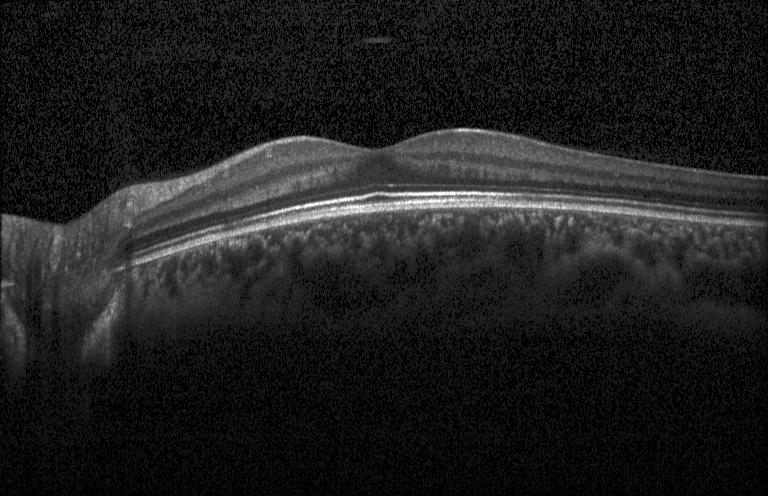

Heidelberg Spectralis OCT system. Macular scan. OCT line scan — Diagnosis: no CNV, no DME, and no drusen.